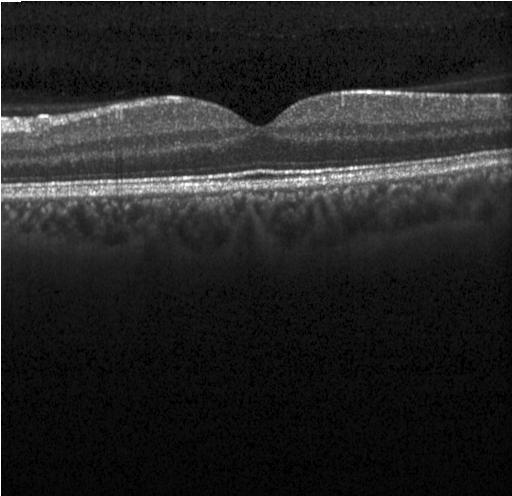
OCT B-scan
No choroidal neovascularization, no diabetic macular edema, and no drusen.